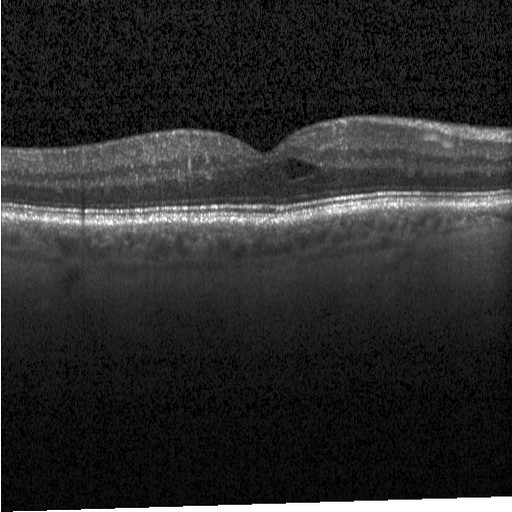 OCT B-scan — Impression: DME.